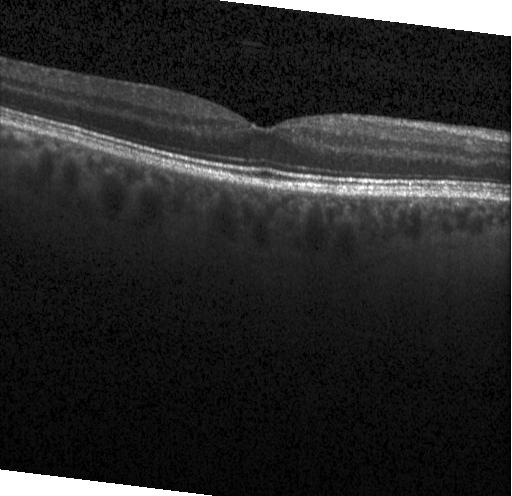
Optical coherence tomography B-scan.
Finding: no choroidal neovascularization, diabetic macular edema, or drusen.